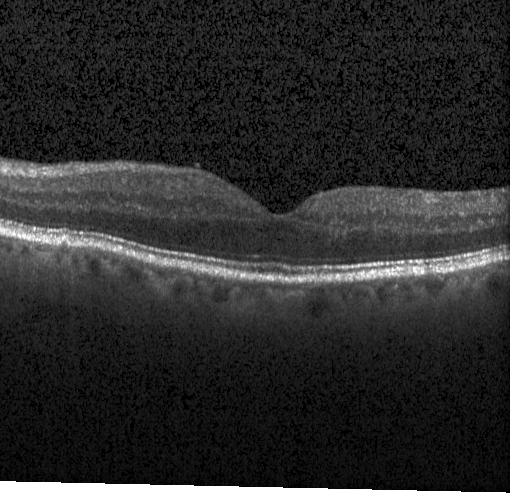

The scan shows neither choroidal neovascularization, diabetic macular edema, nor drusen.